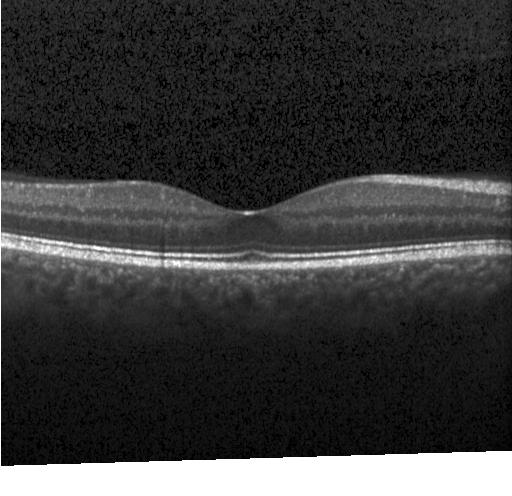 Impression: no choroidal neovascularization, no diabetic macular edema, and no drusen.